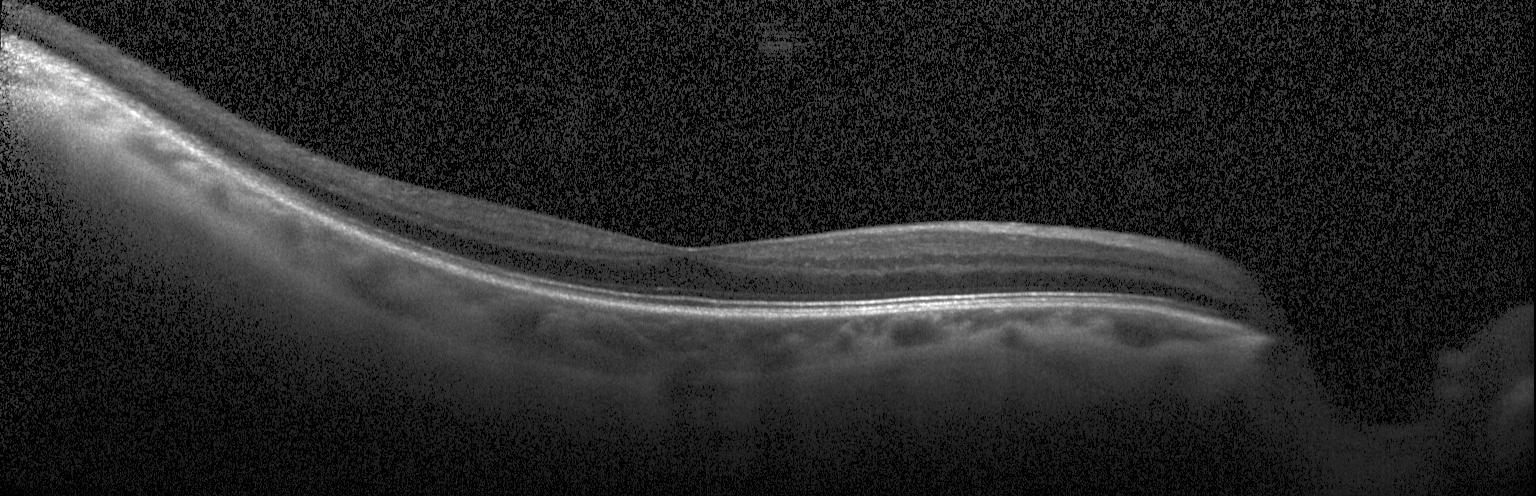

Macular scan · OCT B-scan
Diagnosis: no CNV, DME, or drusen.